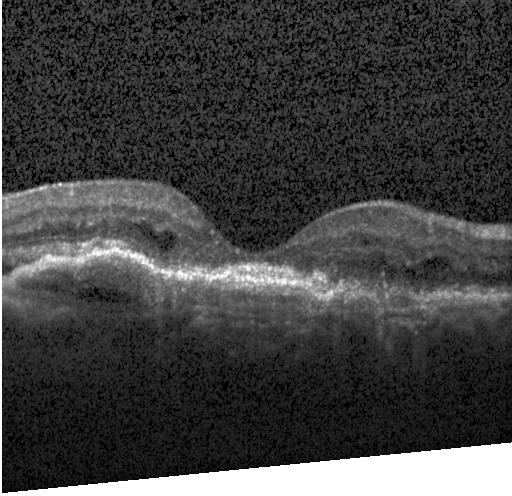
Macular scan, retinal OCT B-scan, spectral-domain OCT, acquired on a Heidelberg Spectralis
Finding: a choroidal neovascular membrane.